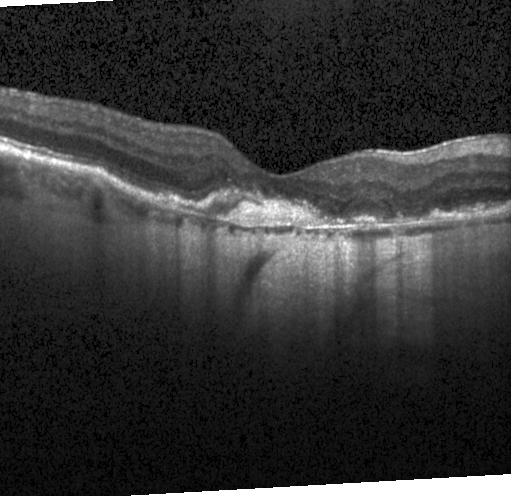
SD-OCT. OCT B-scan. Acquired on a Heidelberg Spectralis. This B-scan demonstrates a choroidal neovascular membrane.